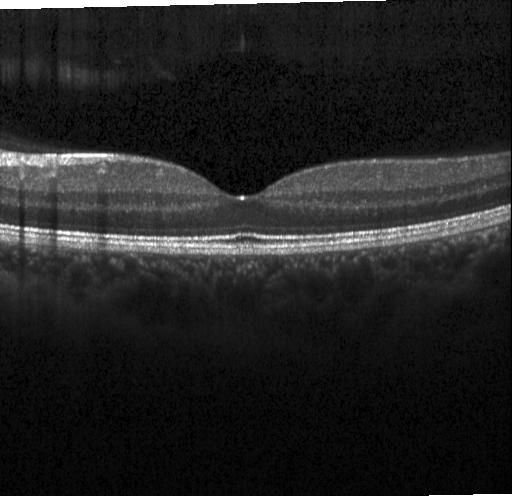

Retinal OCT cross-section; macular scan; spectral-domain optical coherence tomography — OCT finding: no choroidal neovascularization, no diabetic macular edema, and no drusen.